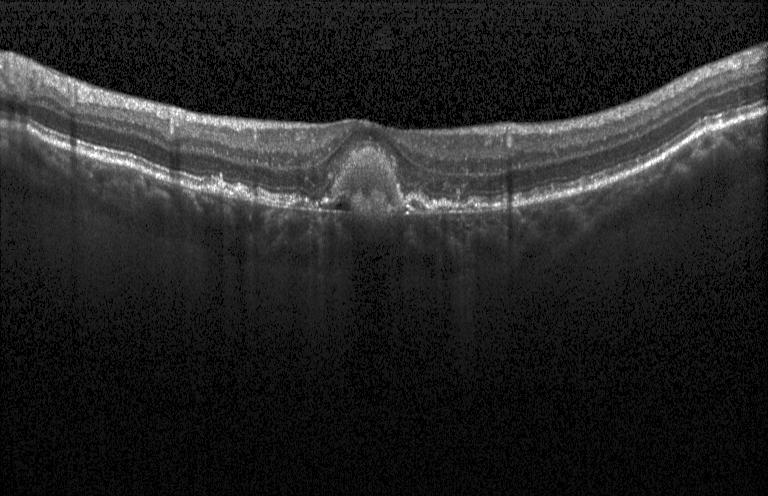 Finding: a choroidal neovascular membrane.